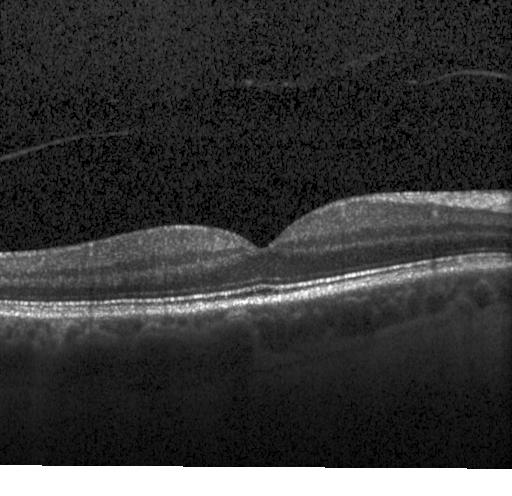
Through the macula; acquired on a Heidelberg Spectralis; retinal OCT cross-section.
Impression: no evidence of choroidal neovascularization, diabetic macular edema, or drusen.